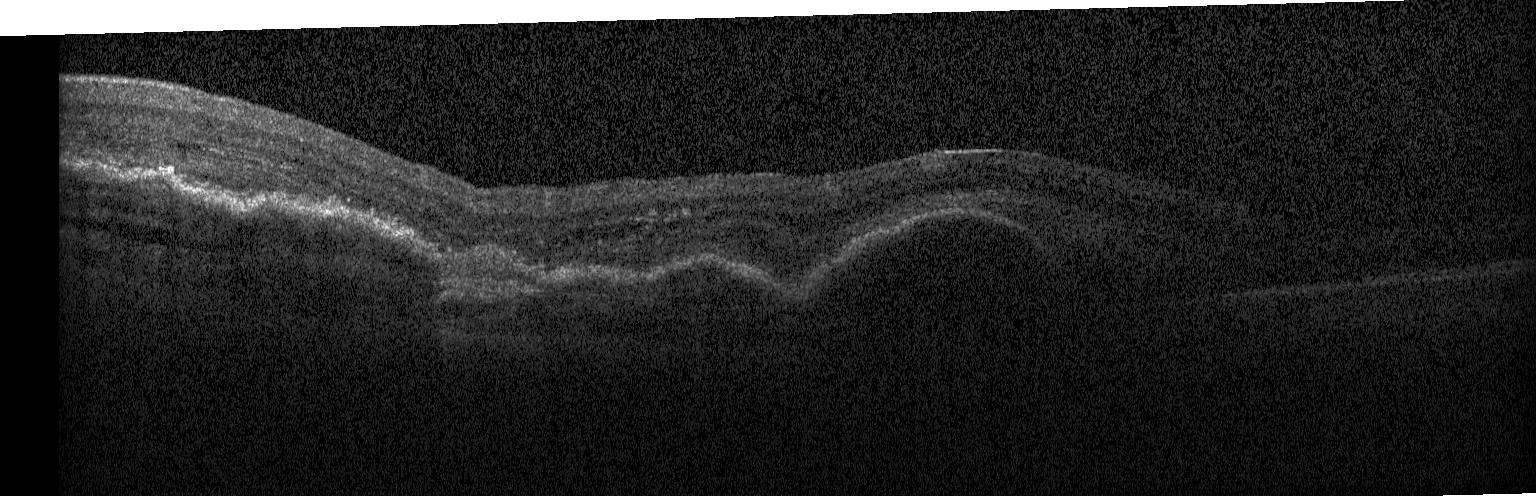
OCT line scan. Dx: choroidal neovascularization.